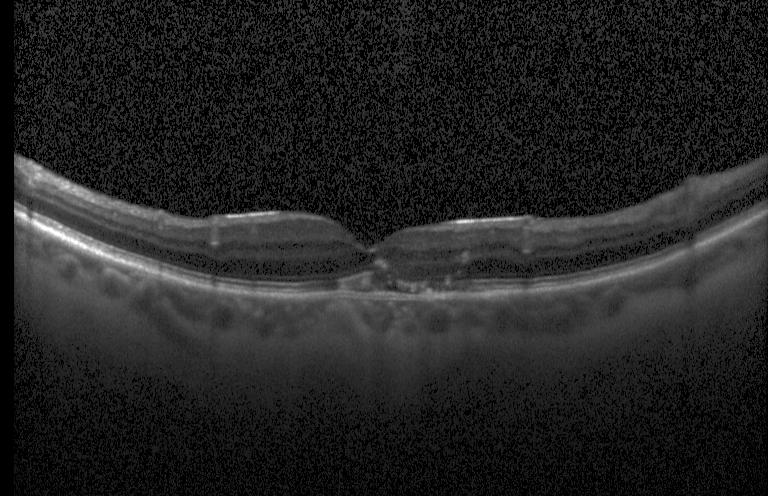
Finding: CNV.